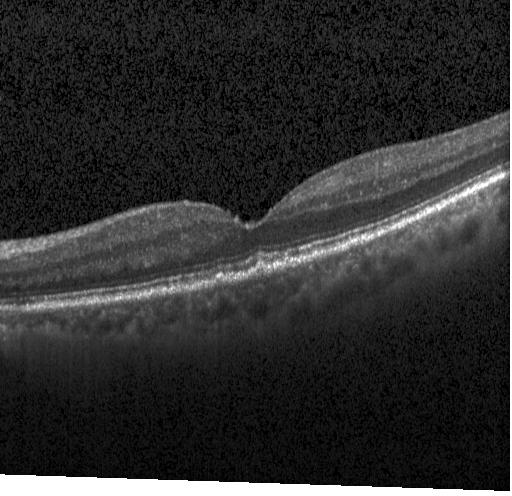 OCT B-scan; SD-OCT; Heidelberg Spectralis. Multiple drusen.